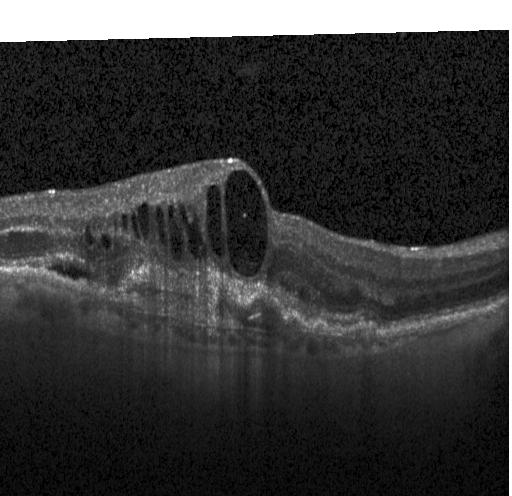

Assessment: a choroidal neovascular membrane.